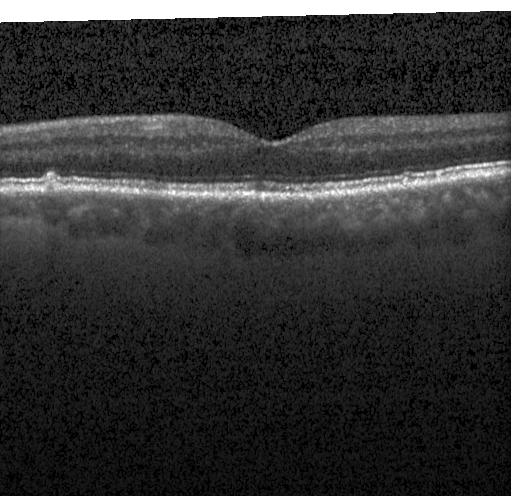

Optical coherence tomography scan
Finding: sub-RPE drusenoid deposits.